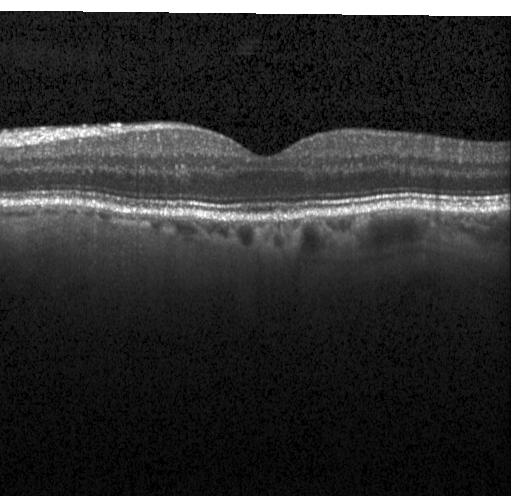
OCT line scan · SD-OCT — This B-scan demonstrates no evidence of choroidal neovascularization, diabetic macular edema, or drusen.